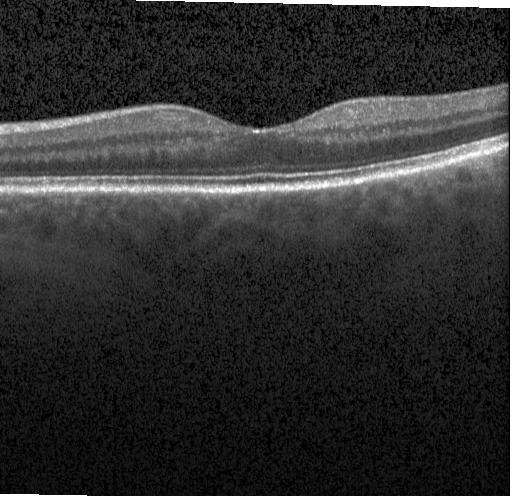
Optical coherence tomography B-scan.
The scan shows no choroidal neovascularization, no diabetic macular edema, and no drusen.